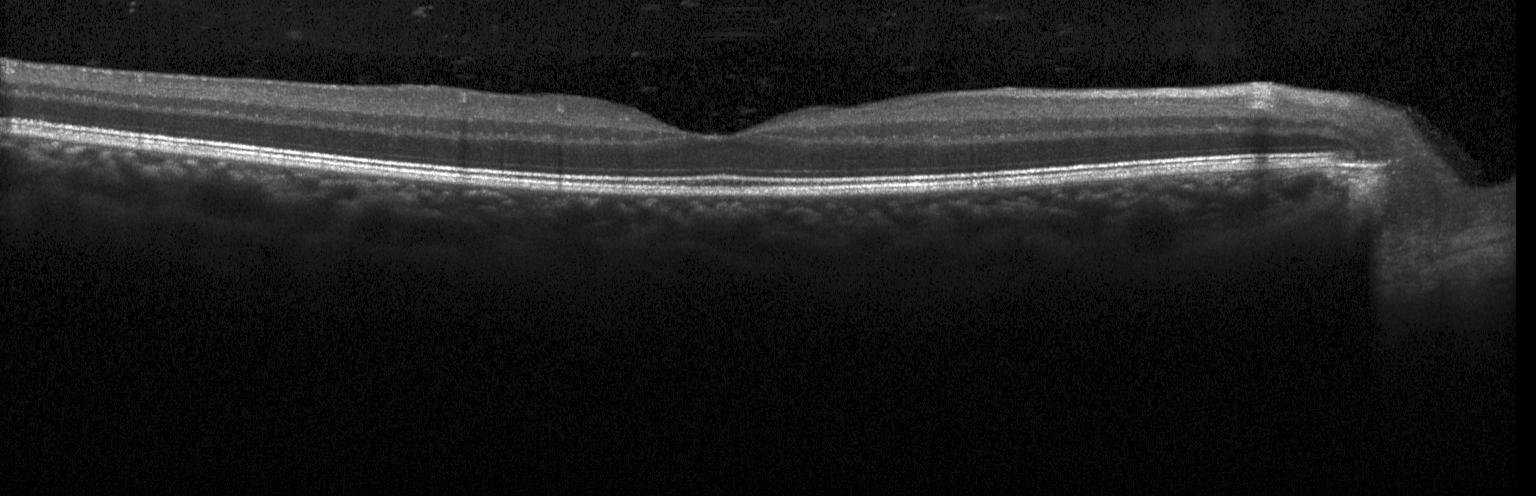 Optical coherence tomography B-scan — Impression: no choroidal neovascularization, no diabetic macular edema, and no drusen.